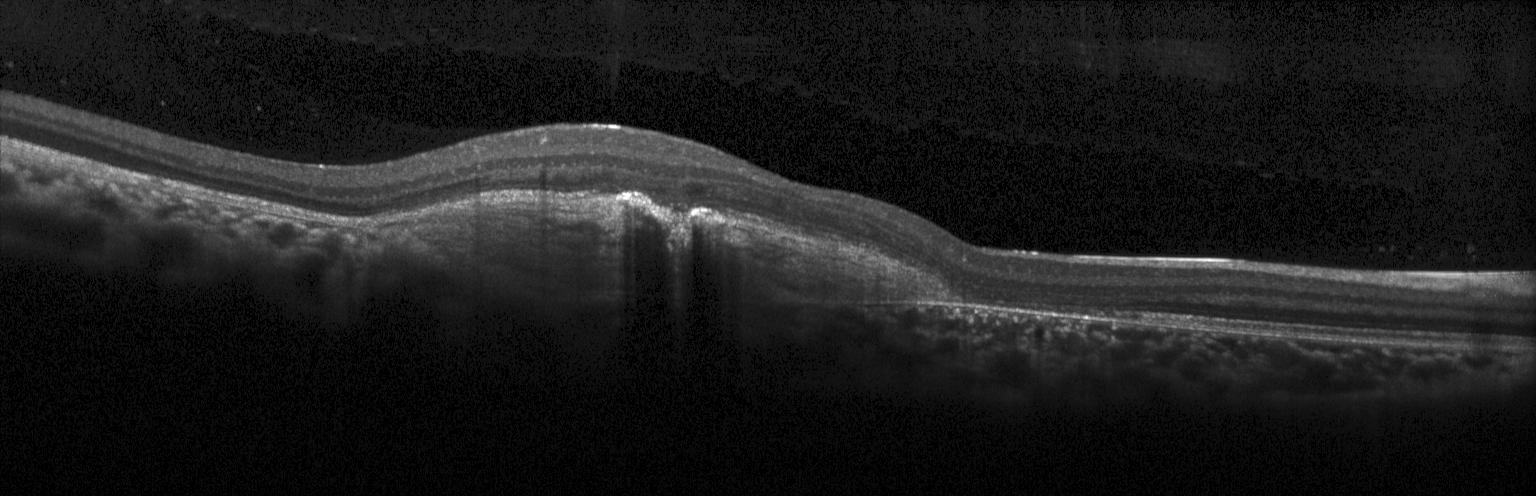 Retinal OCT cross-section showing choroidal neovascularization (CNV).